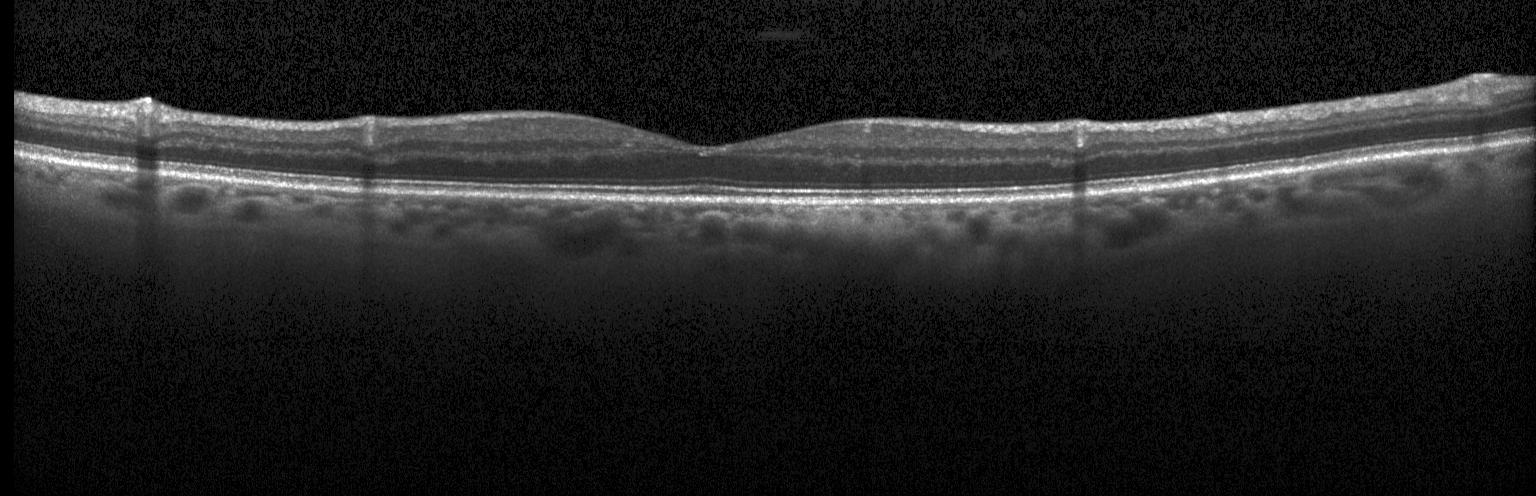 Retinal OCT cross-section.
Finding: no CNV, DME, or drusen.